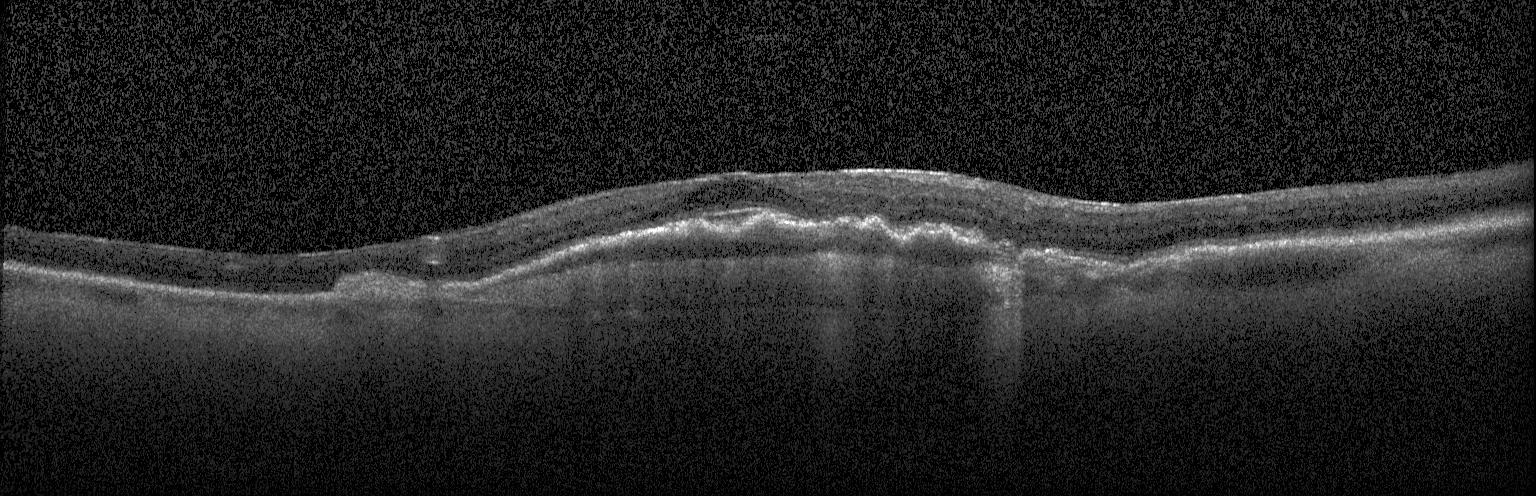 Heidelberg Spectralis OCT system. Through the macula. SD-OCT. Optical coherence tomography scan — This B-scan demonstrates choroidal neovascularization.